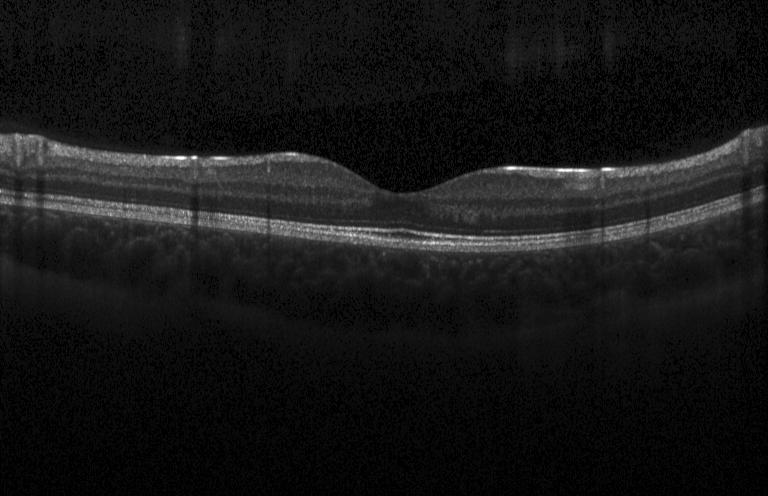

OCT B-scan · spectral-domain OCT · fovea-centered. Finding: neither choroidal neovascularization, diabetic macular edema, nor drusen.